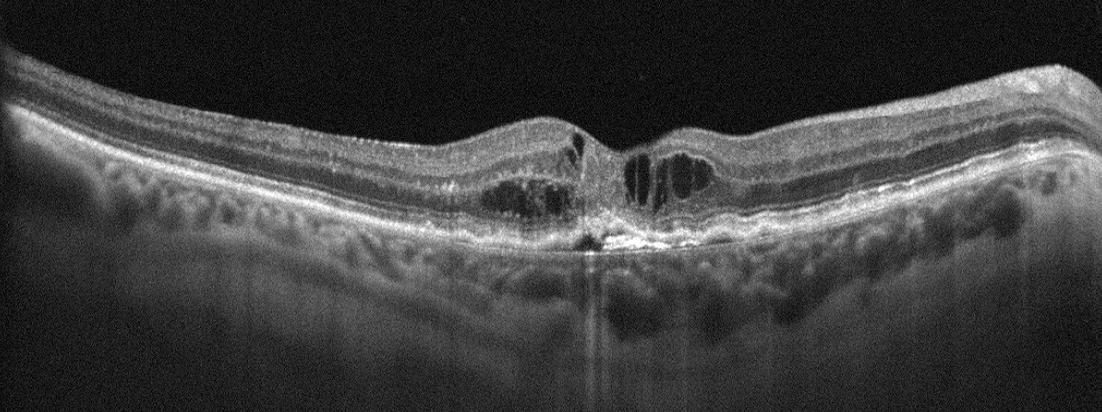
Retinal OCT B-scan; through the macula. Finding: age-related macular degeneration.